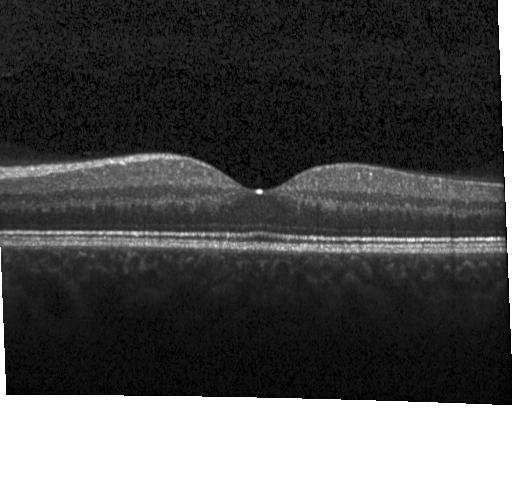 Fovea-centered · optical coherence tomography B-scan
Finding: no CNV, DME, or drusen.